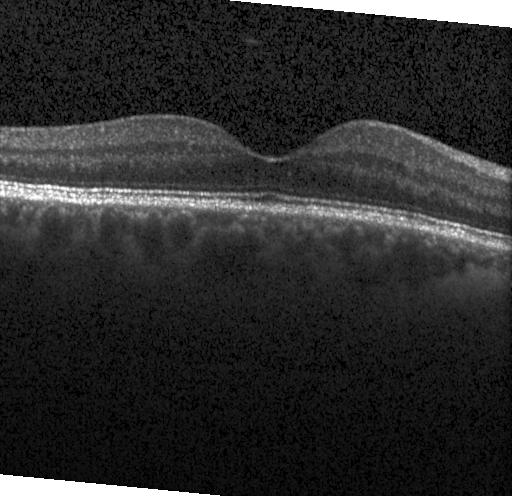

Retinal OCT cross-section showing no evidence of choroidal neovascularization, diabetic macular edema, or drusen.